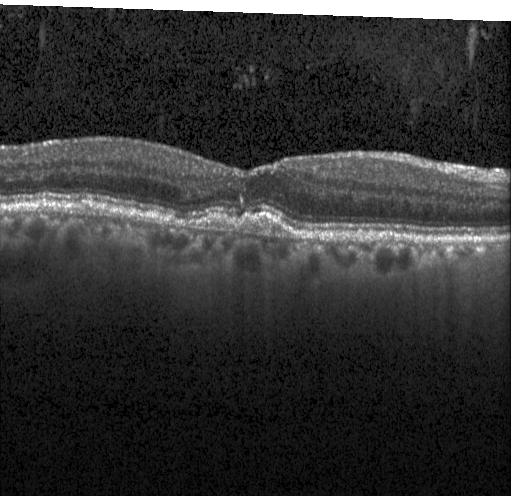
This B-scan demonstrates a choroidal neovascular membrane.